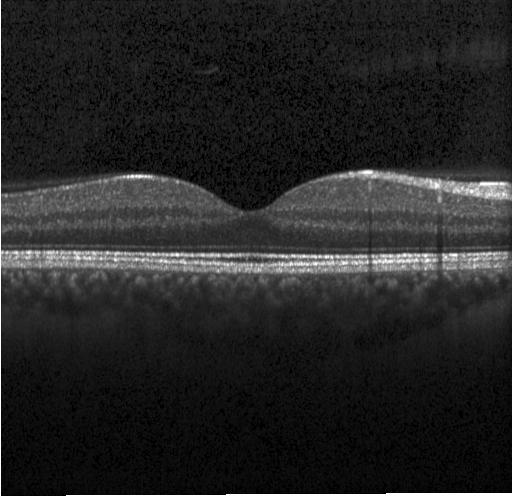
OCT line scan. No evidence of choroidal neovascularization, diabetic macular edema, or drusen.